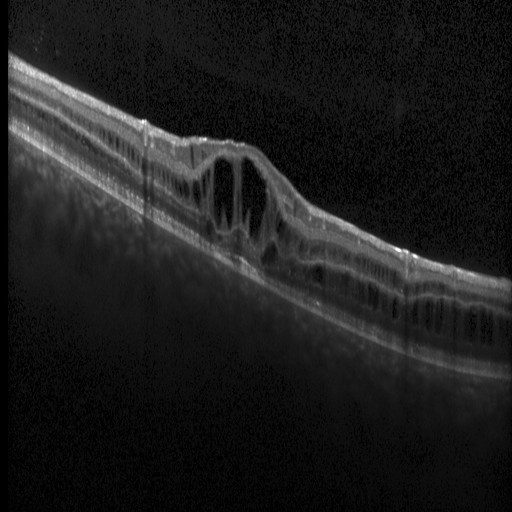
SD-OCT; instrument: Heidelberg Spectralis; through the macula; optical coherence tomography scan — OCT finding: diabetic macular edema (DME).